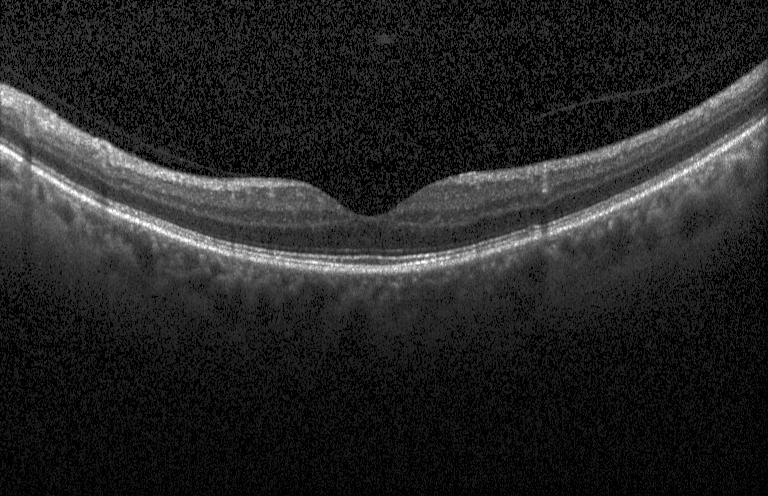 Horizontal scan through the fovea, Heidelberg Spectralis, retinal OCT B-scan — OCT finding: no choroidal neovascularization, no diabetic macular edema, and no drusen.